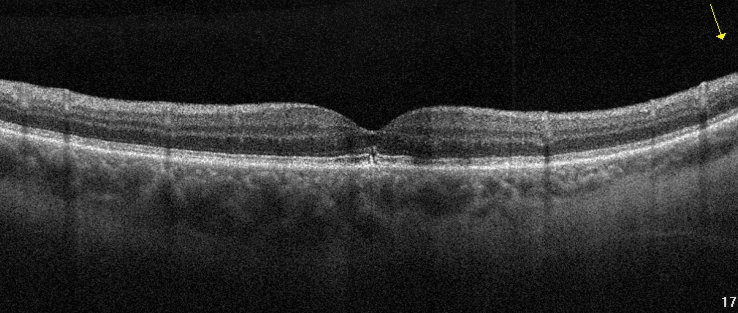

Impression: AMD.